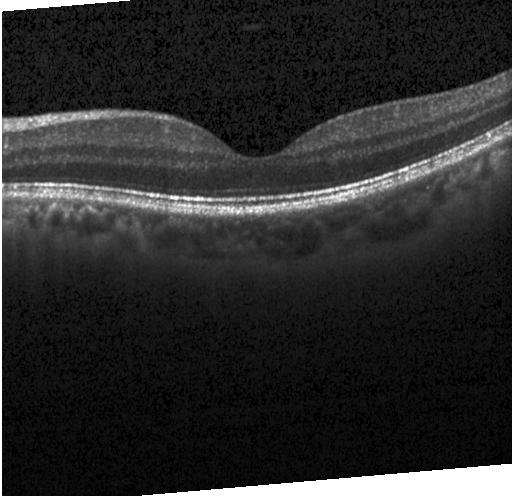

This B-scan demonstrates no evidence of CNV, DME, or drusen.